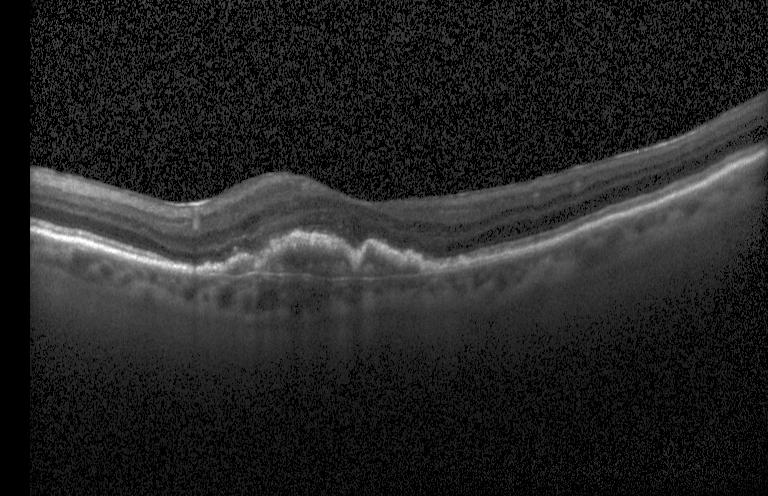
Acquired on a Heidelberg Spectralis; spectral-domain optical coherence tomography; retinal OCT B-scan; fovea-centered — Dx: choroidal neovascularization.